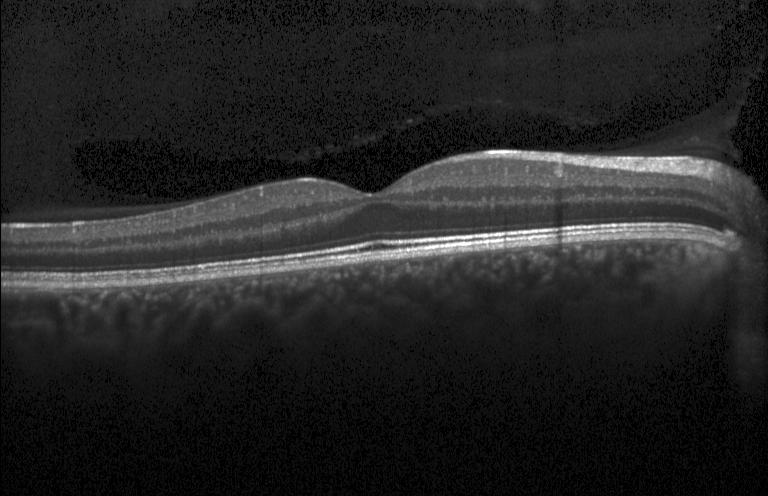
Macular OCT demonstrating no choroidal neovascularization, no diabetic macular edema, and no drusen.